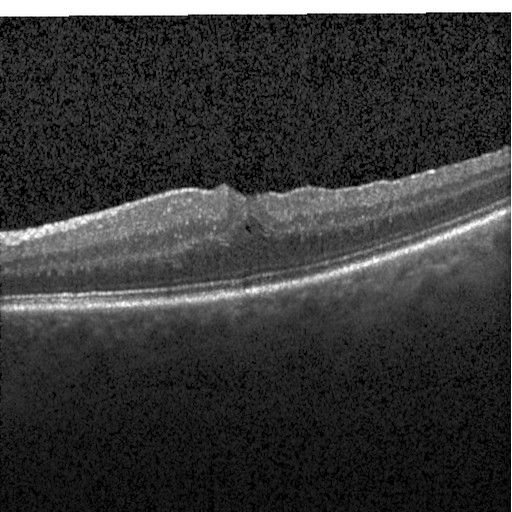
Retinal OCT cross-section, Heidelberg Spectralis, spectral-domain optical coherence tomography — Finding: diabetic macular edema (DME).